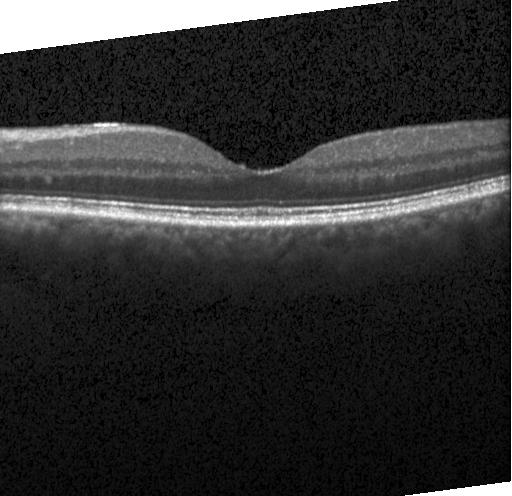 Retinal OCT B-scan
Impression: no choroidal neovascularization, no diabetic macular edema, and no drusen.